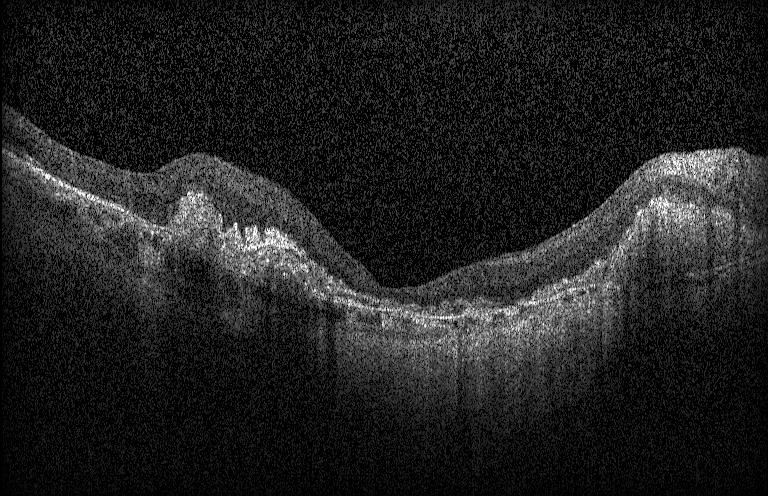 Spectral-domain OCT B-scan: choroidal neovascularization (CNV).